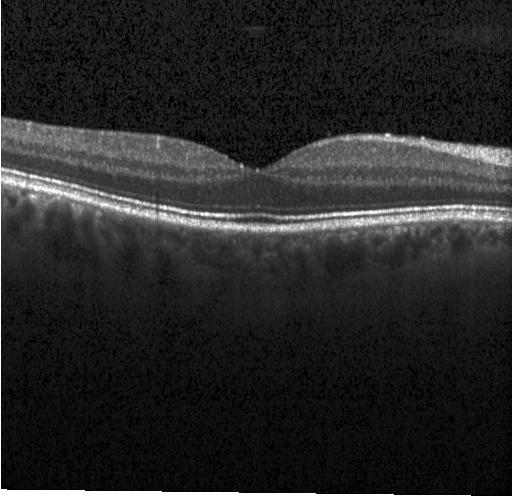

OCT line scan · instrument: Heidelberg Spectralis · SD-OCT · horizontal scan through the fovea
Dx: no CNV, DME, or drusen.